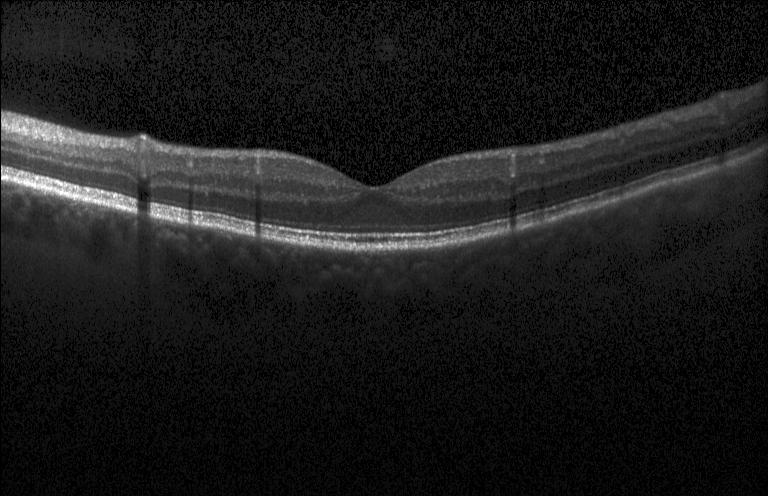
Heidelberg Spectralis. Retinal OCT cross-section — This B-scan demonstrates no evidence of choroidal neovascularization, diabetic macular edema, or drusen.